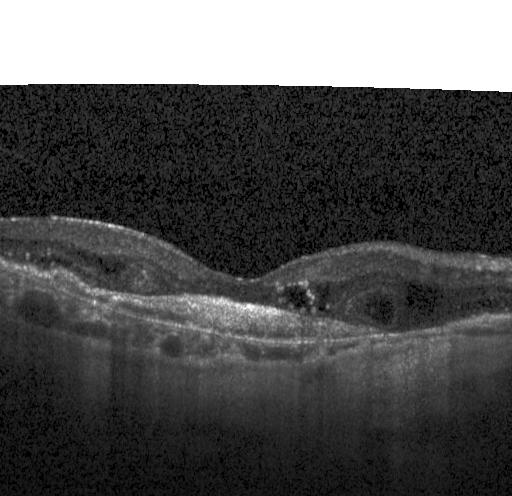

Retinal OCT cross-section.
This B-scan demonstrates choroidal neovascularization (CNV).